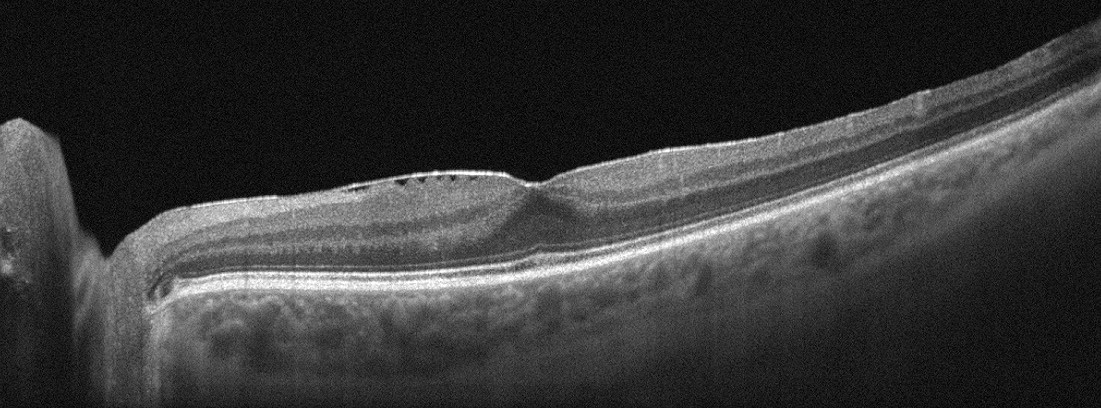 Macular scan · retinal OCT B-scan — Epiretinal membrane.